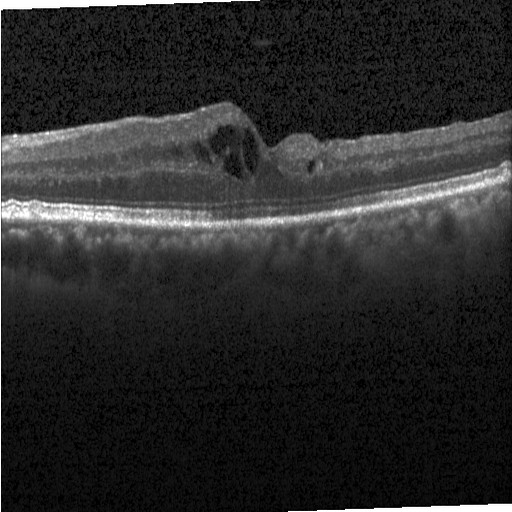

Optical coherence tomography B-scan — Finding: DME.